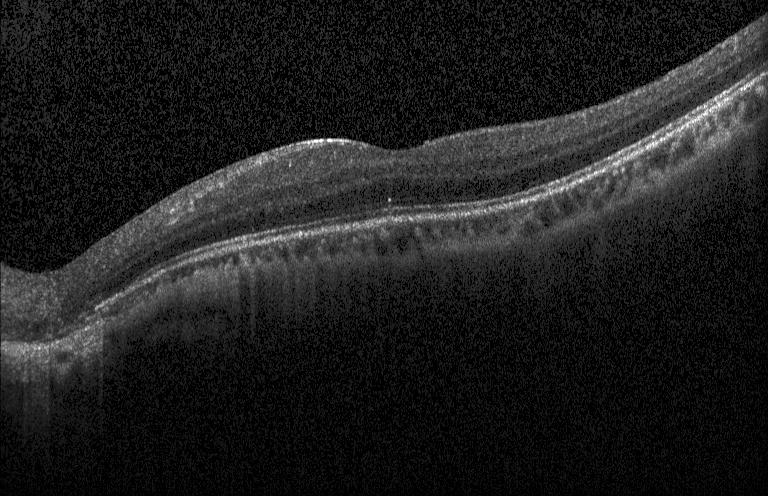 Horizontal scan through the fovea; instrument: Heidelberg Spectralis; retinal OCT B-scan; SD-OCT. Assessment: no CNV, no DME, and no drusen.